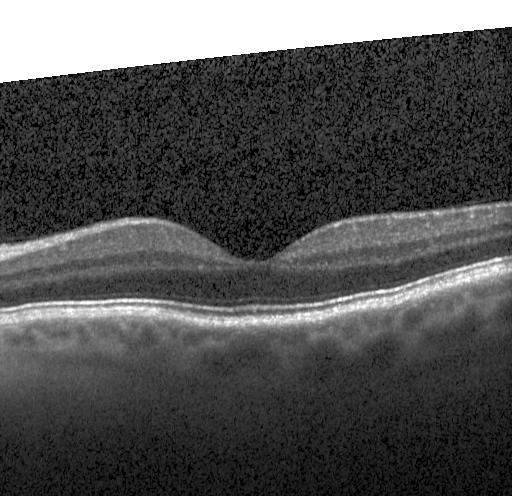
Optical coherence tomography scan; Heidelberg Spectralis OCT system
The scan shows no CNV, no DME, and no drusen.